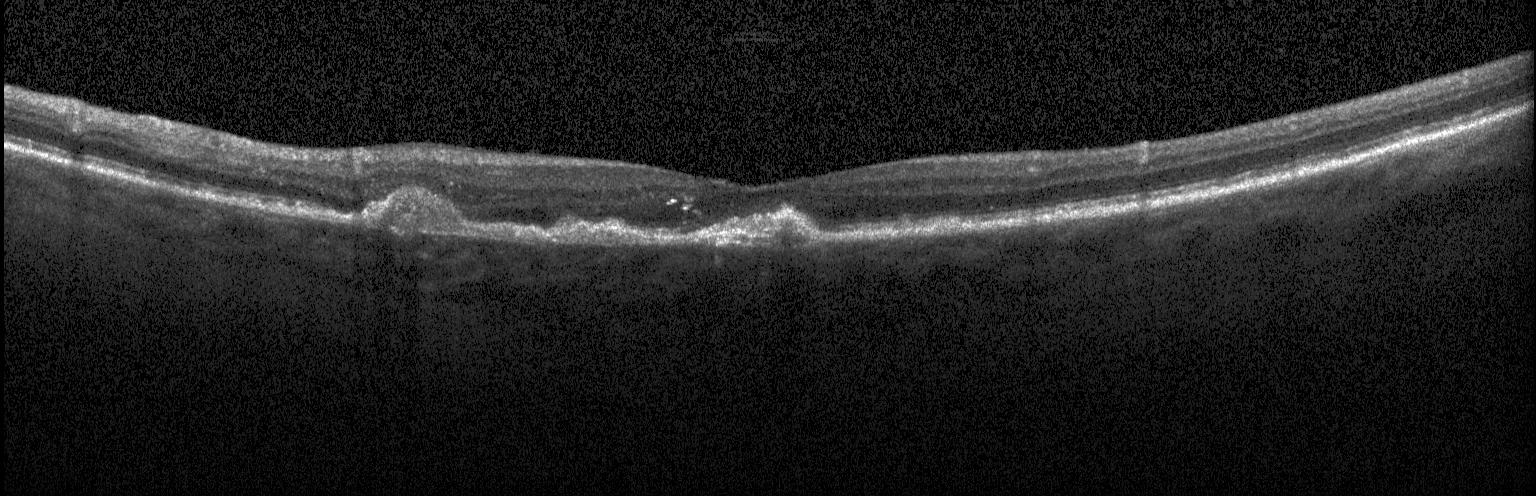

Spectral-domain OCT, acquired on a Heidelberg Spectralis, retinal OCT B-scan — OCT finding: a choroidal neovascular membrane.